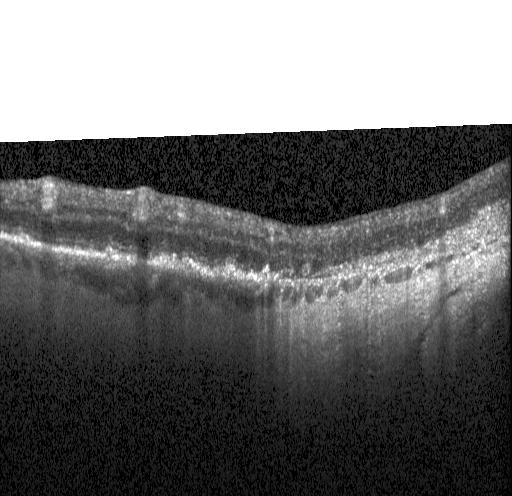
OCT B-scan
Impression: choroidal neovascularization.